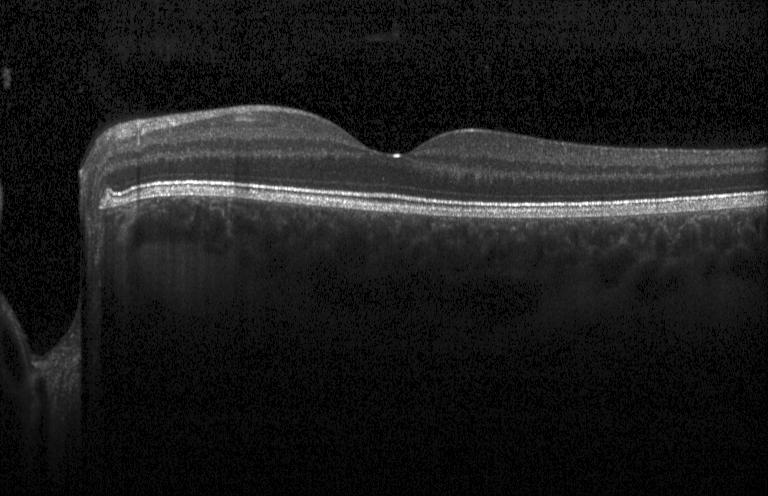

Retinal OCT cross-section showing no evidence of choroidal neovascularization, diabetic macular edema, or drusen.